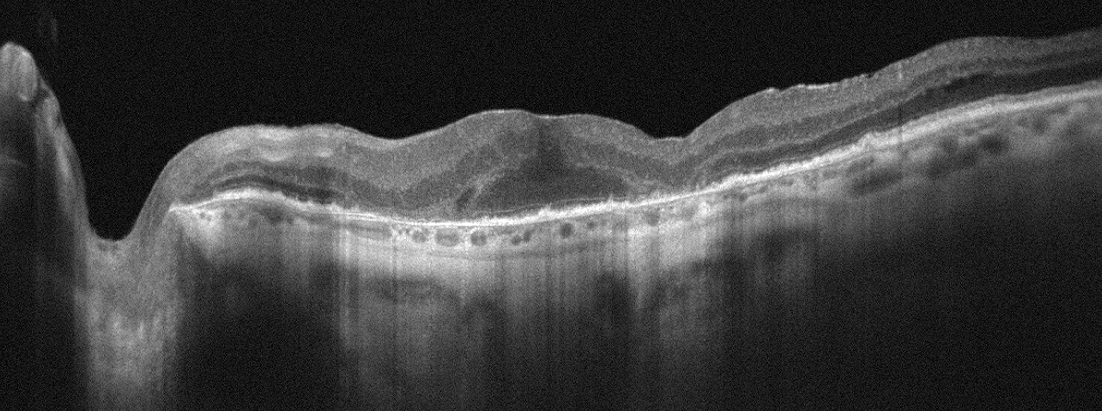
Dx: AMD.